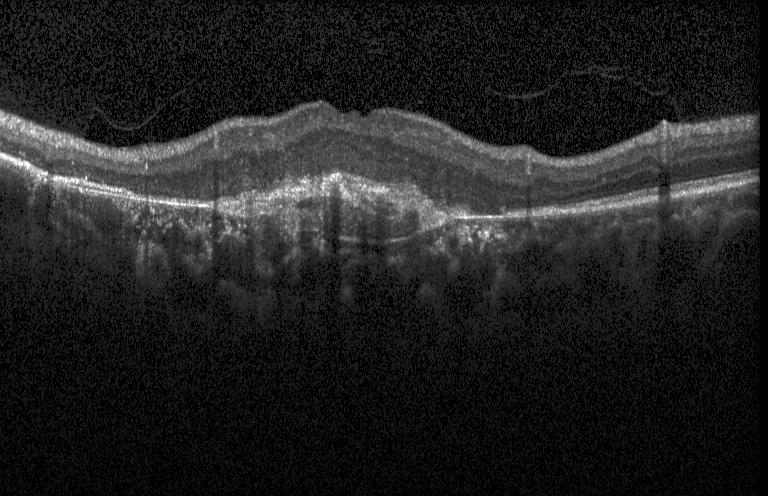
Macular OCT: choroidal neovascularization (CNV).